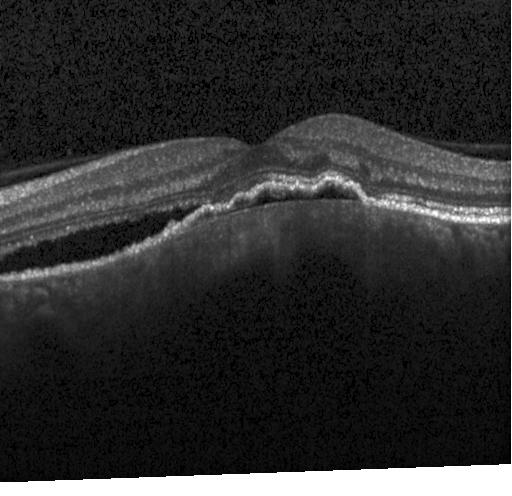

Macular scan, optical coherence tomography scan, acquired on a Heidelberg Spectralis — Impression: a choroidal neovascular membrane.